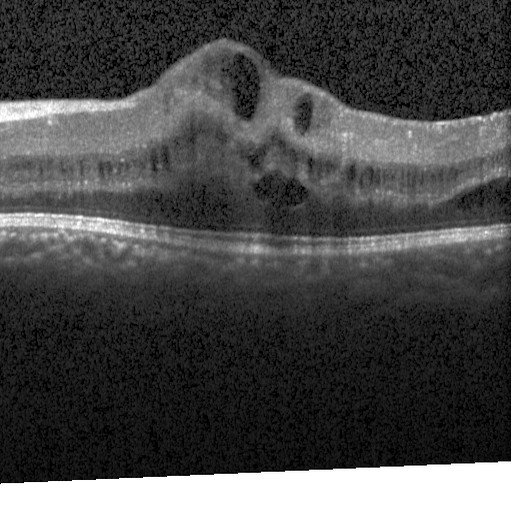 Spectral-domain optical coherence tomography · acquired on a Heidelberg Spectralis · retinal OCT cross-section · fovea-centered
Macular OCT: DME.